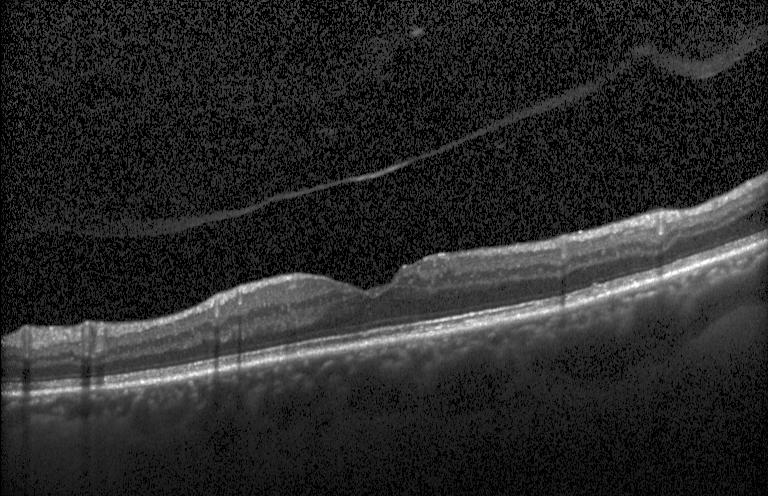

Impression: no evidence of choroidal neovascularization, diabetic macular edema, or drusen.